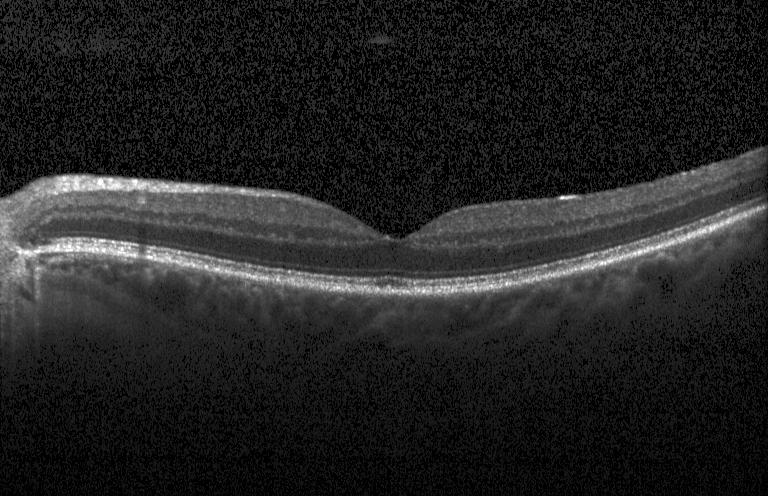 This B-scan demonstrates no choroidal neovascularization, diabetic macular edema, or drusen.